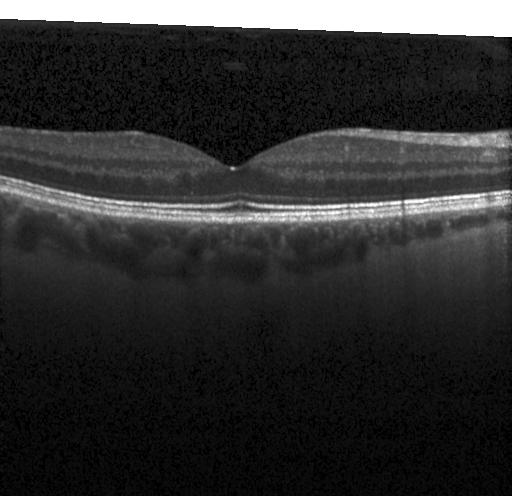 Optical coherence tomography B-scan — OCT finding: no CNV, DME, or drusen.